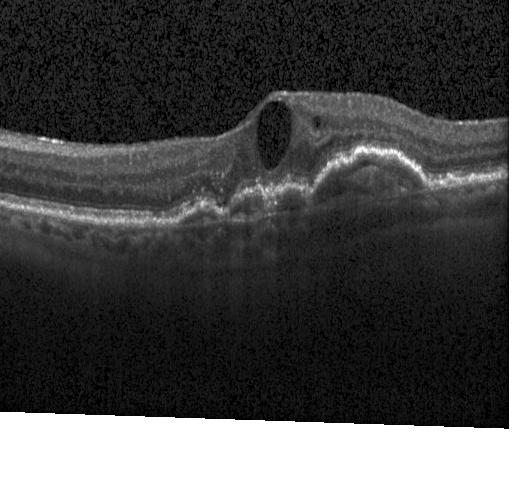

OCT B-scan — Finding: CNV.